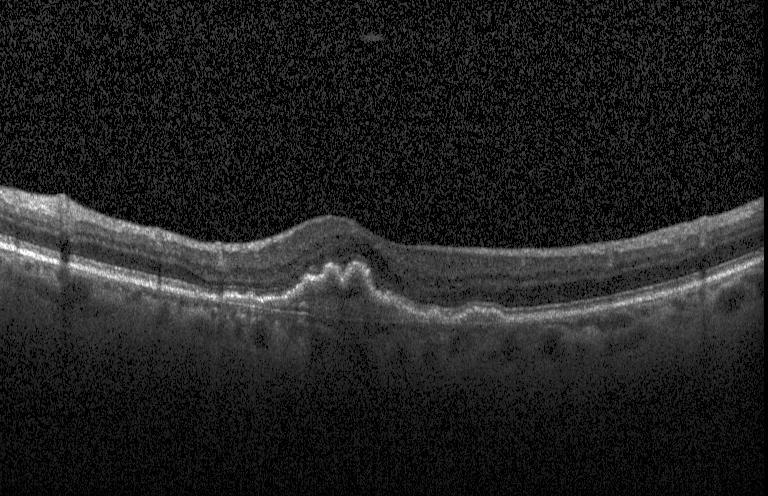
Through the macula, retinal OCT B-scan, spectral-domain OCT — Impression: a choroidal neovascular membrane.